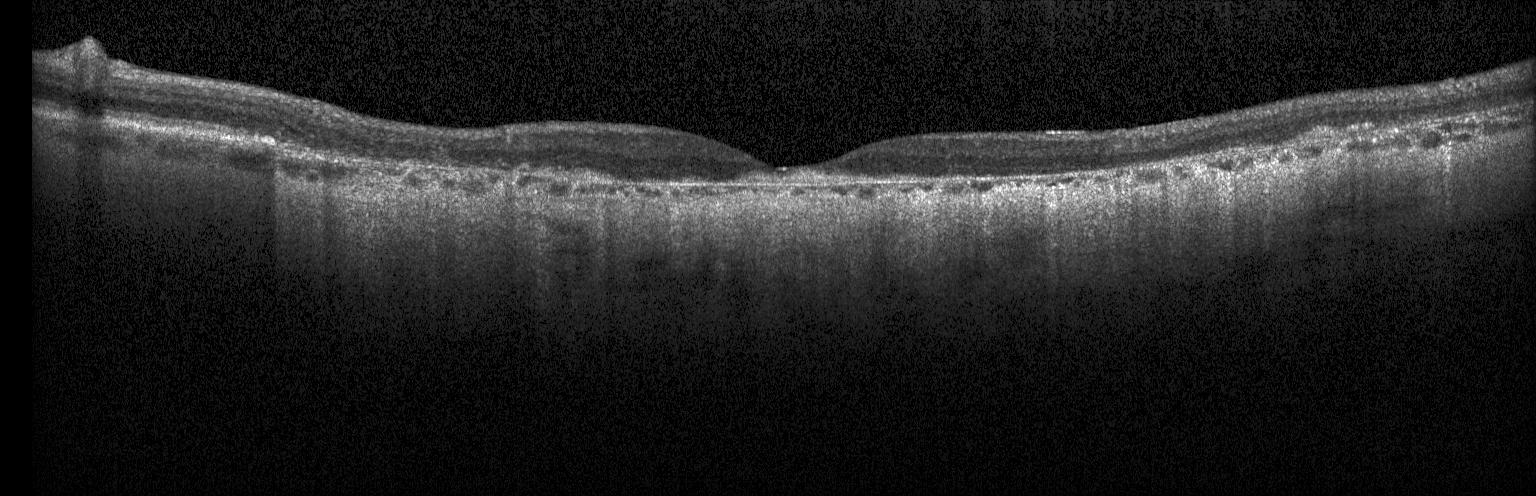
Finding: choroidal neovascularization (CNV).